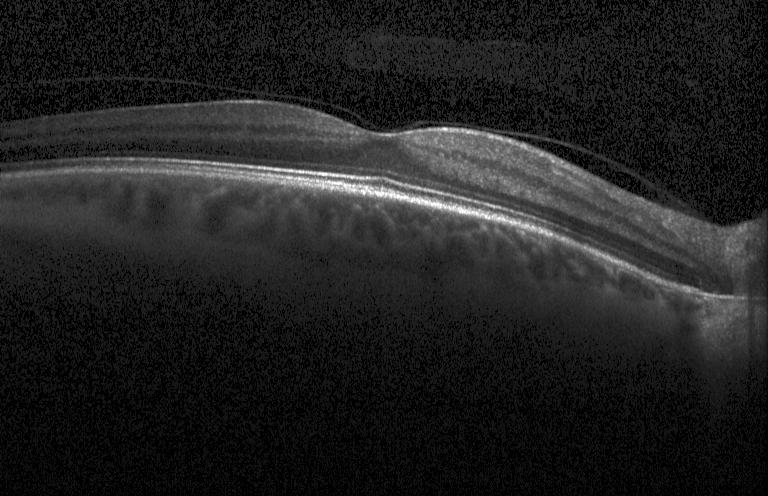
Fovea-centered, instrument: Heidelberg Spectralis, retinal OCT B-scan
OCT finding: no choroidal neovascularization, diabetic macular edema, or drusen.